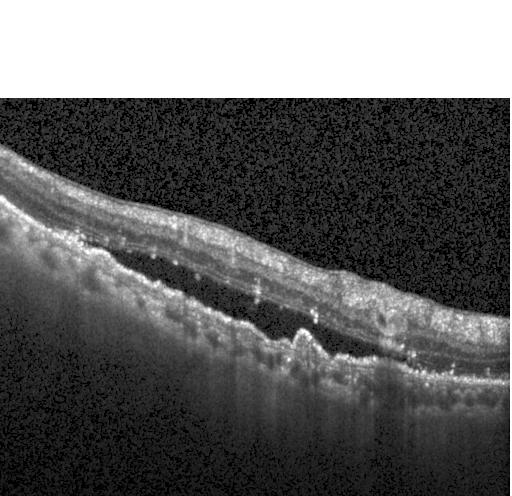
Optical coherence tomography scan; horizontal scan through the fovea. Finding: a choroidal neovascular membrane.